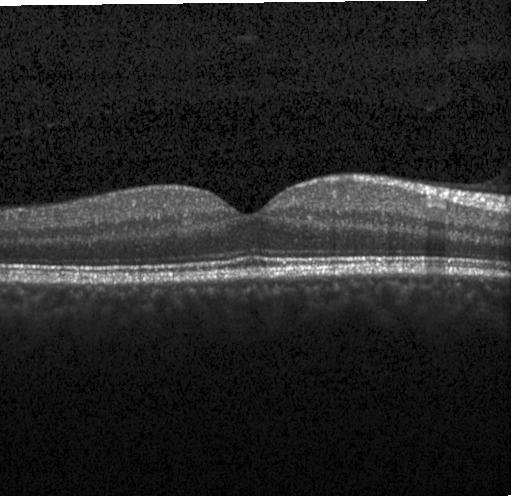 OCT finding: no choroidal neovascularization, diabetic macular edema, or drusen.